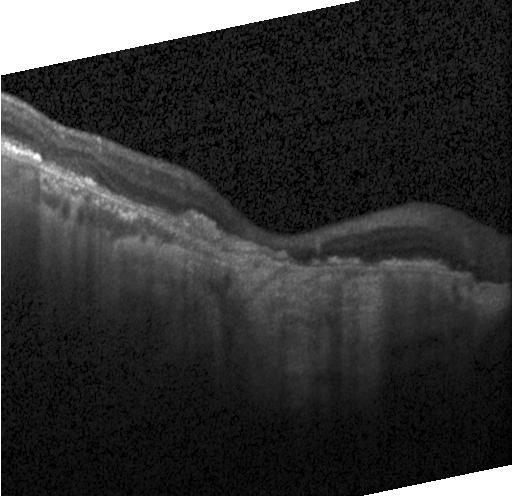

Retinal OCT B-scan. The scan shows a choroidal neovascular membrane.